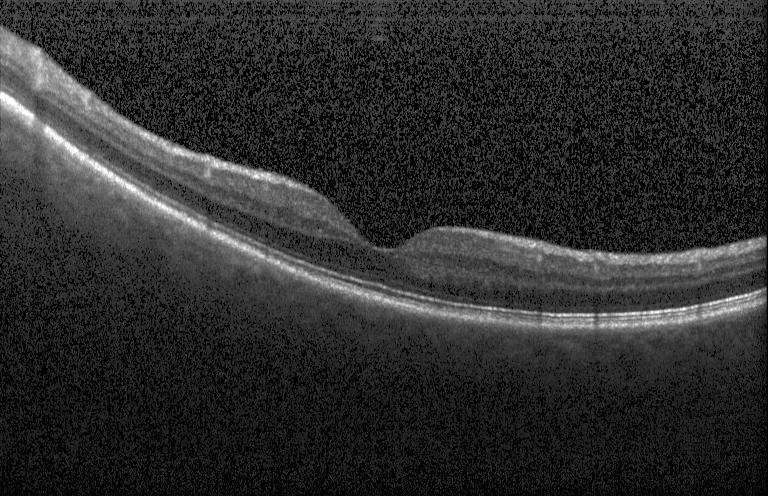 OCT B-scan; centered on the fovea
Impression: no choroidal neovascularization, no diabetic macular edema, and no drusen.